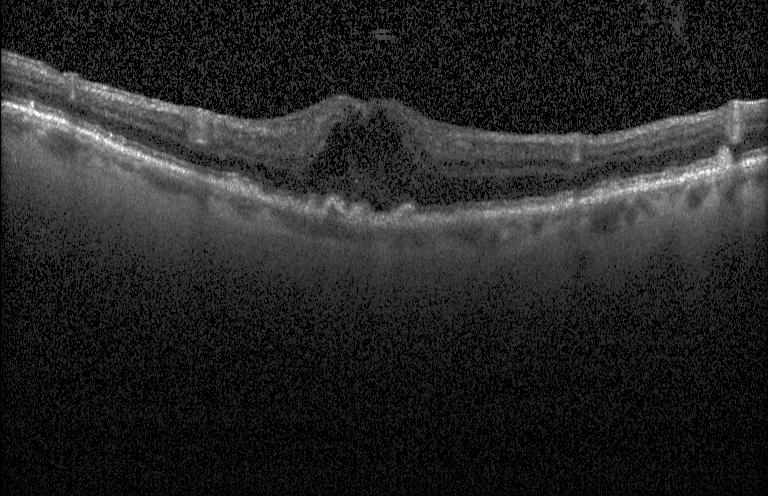 Horizontal scan through the fovea. Spectral-domain OCT. OCT B-scan. Heidelberg Spectralis.
Impression: choroidal neovascularization.